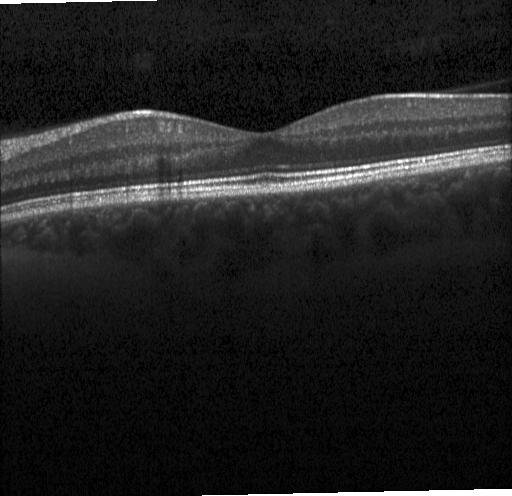 Macular OCT demonstrating neither choroidal neovascularization, diabetic macular edema, nor drusen.